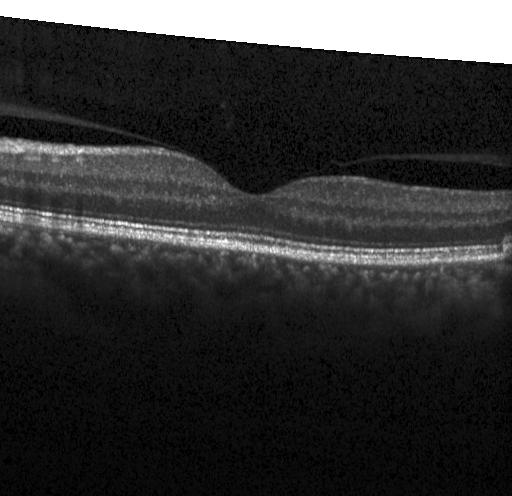
Diagnosis: no choroidal neovascularization, no diabetic macular edema, and no drusen.